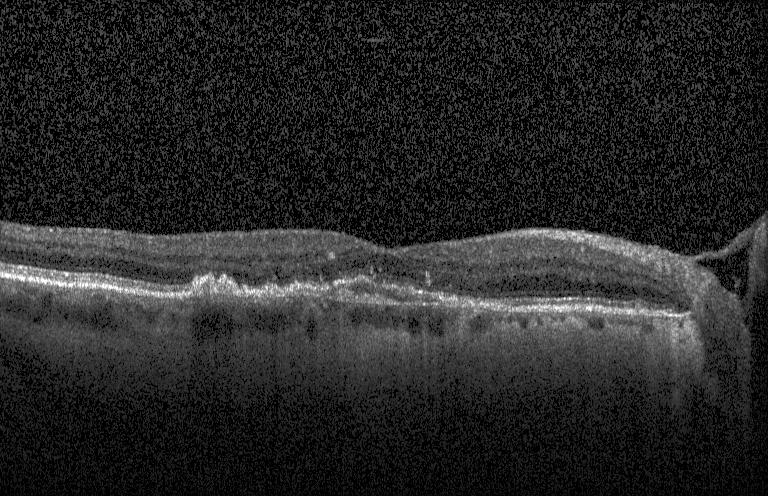

SD-OCT, retinal OCT B-scan.
Assessment: a choroidal neovascular membrane.